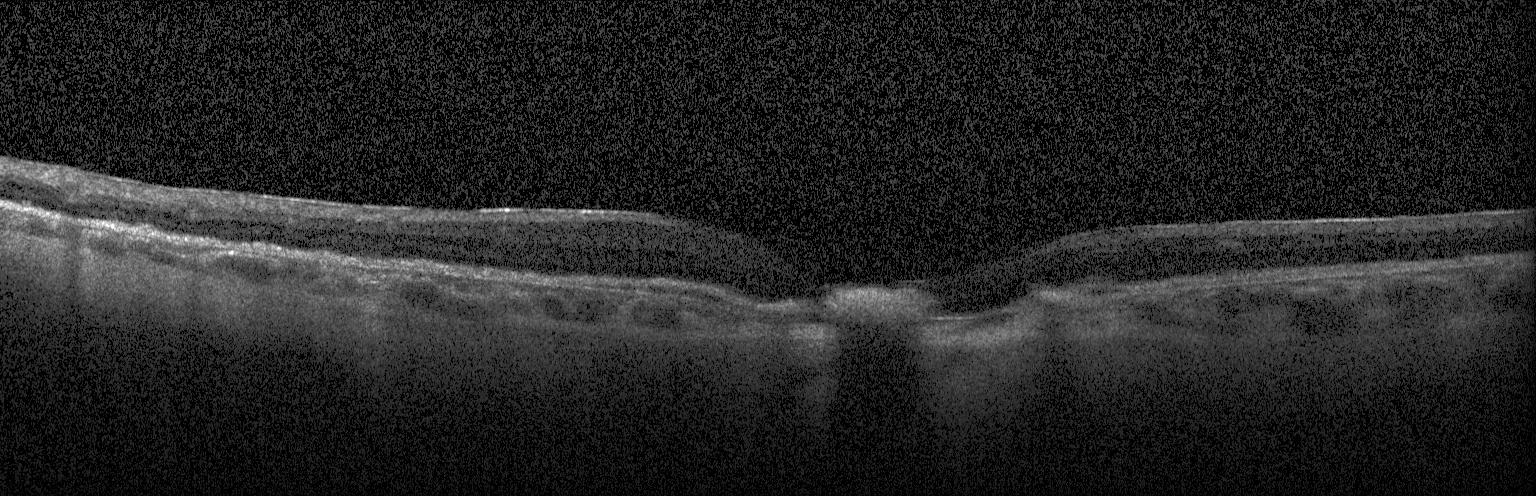

Retinal OCT cross-section; Heidelberg Spectralis; through the macula; spectral-domain optical coherence tomography — Macular OCT: a choroidal neovascular membrane.